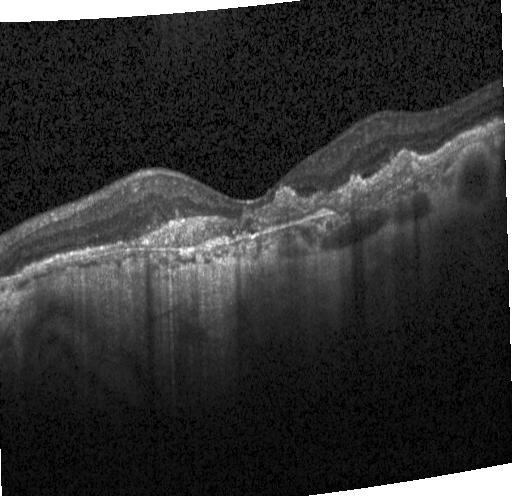

Macular OCT: a choroidal neovascular membrane.